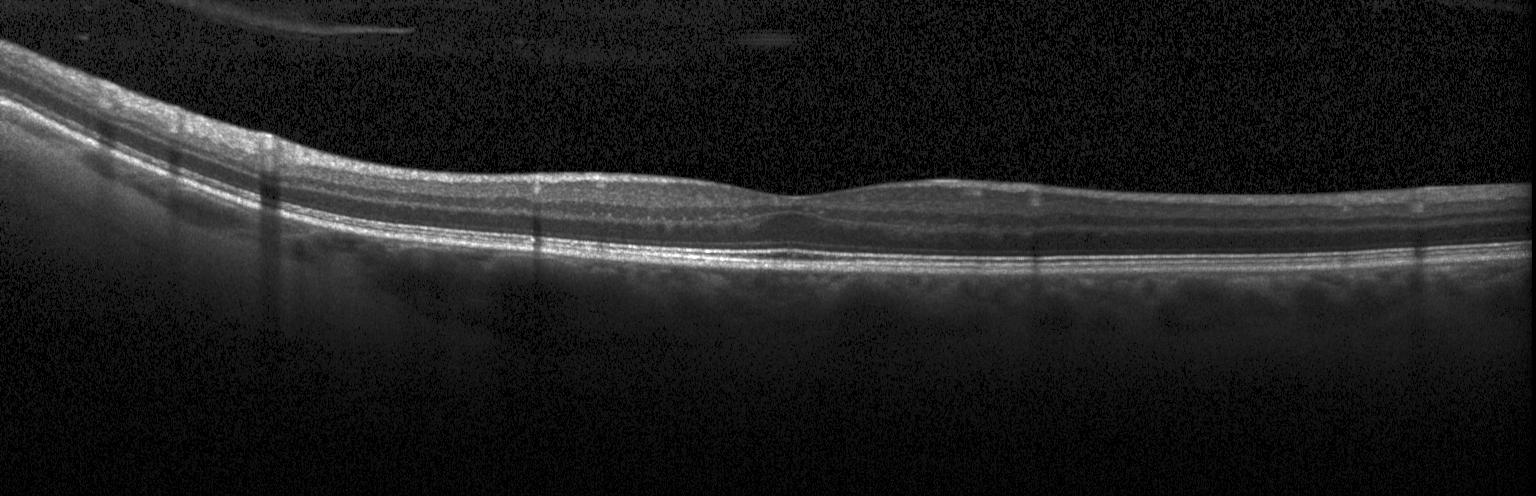 Optical coherence tomography B-scan — Finding: no choroidal neovascularization, no diabetic macular edema, and no drusen.